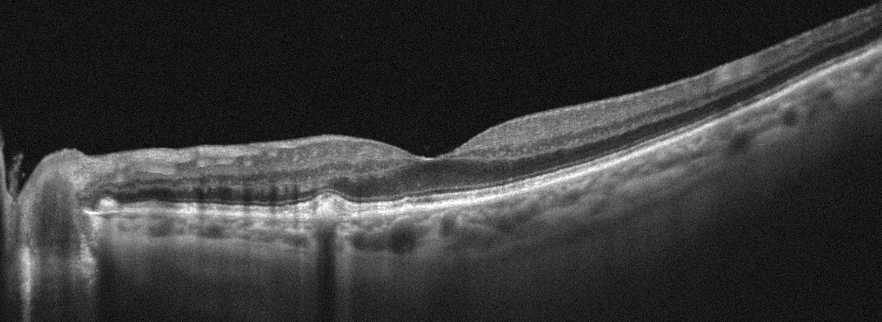
OCT line scan. OS
This B-scan demonstrates age-related macular degeneration.